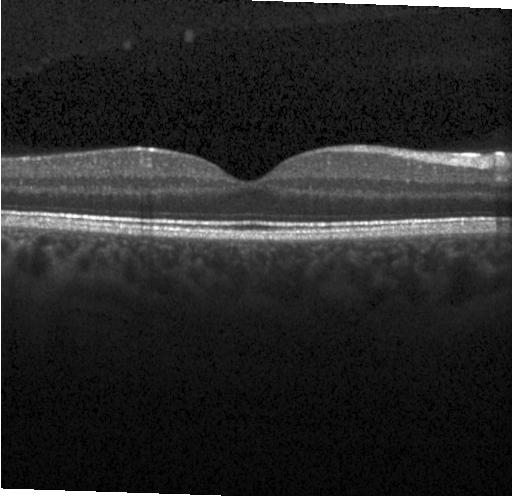 Macular OCT: no CNV, no DME, and no drusen.